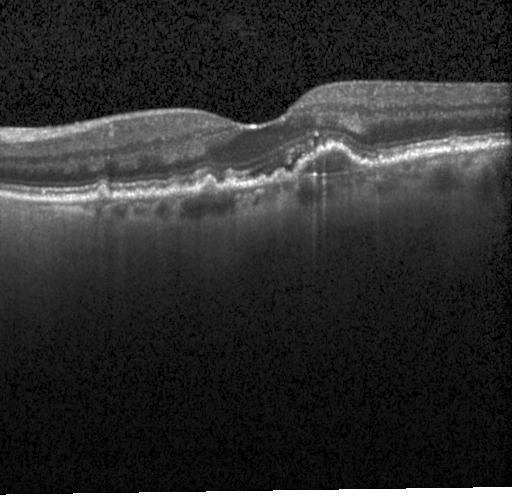 Impression: choroidal neovascularization (CNV).